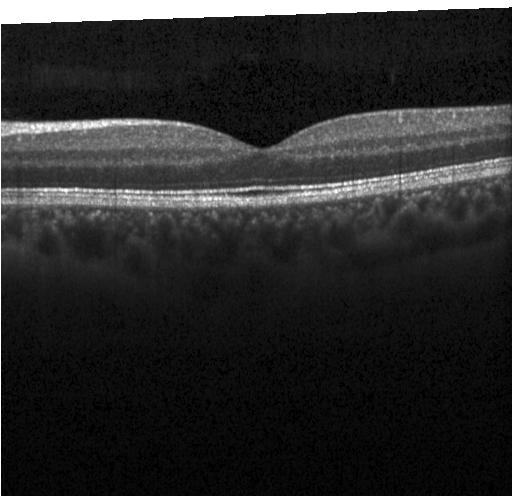 Impression: no choroidal neovascularization, no diabetic macular edema, and no drusen.